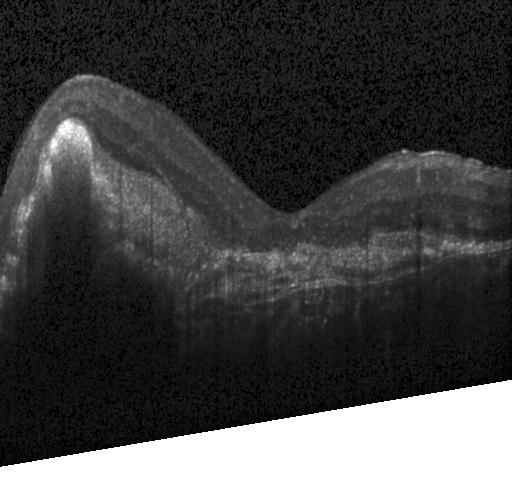
Retinal OCT cross-section, spectral-domain optical coherence tomography. The scan shows a choroidal neovascular membrane.